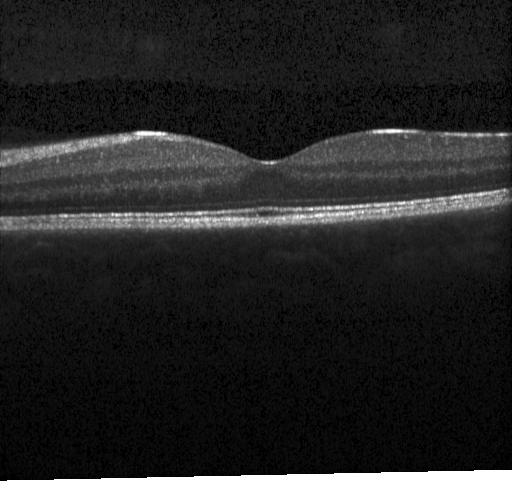
Optical coherence tomography B-scan · through the macula — OCT finding: no evidence of choroidal neovascularization, diabetic macular edema, or drusen.